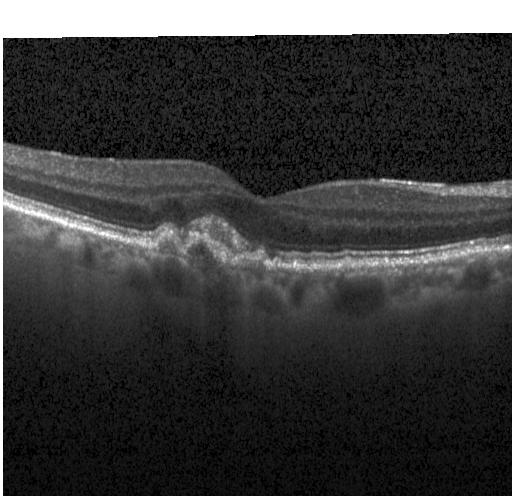

OCT line scan · spectral-domain OCT — Assessment: CNV.